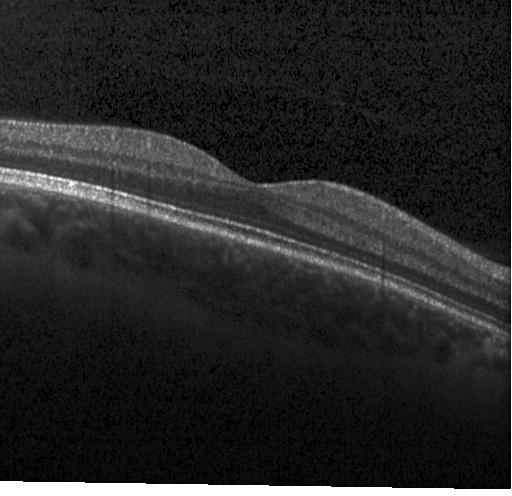 Retinal OCT cross-section showing neither choroidal neovascularization, diabetic macular edema, nor drusen.